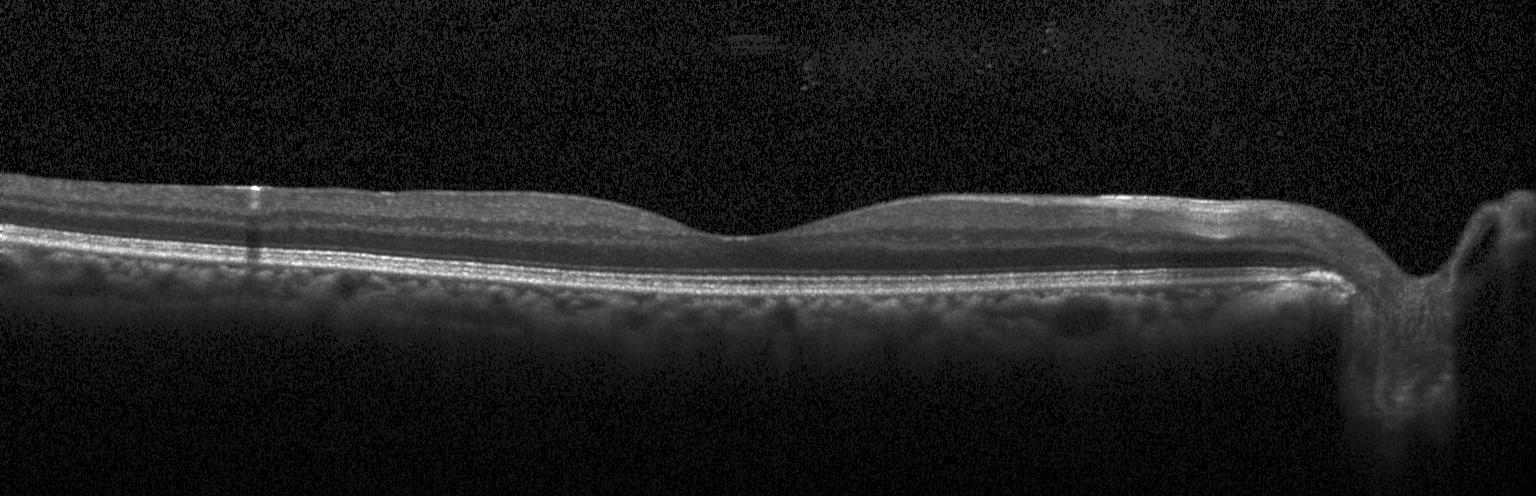
OCT line scan.
This B-scan demonstrates no CNV, no DME, and no drusen.